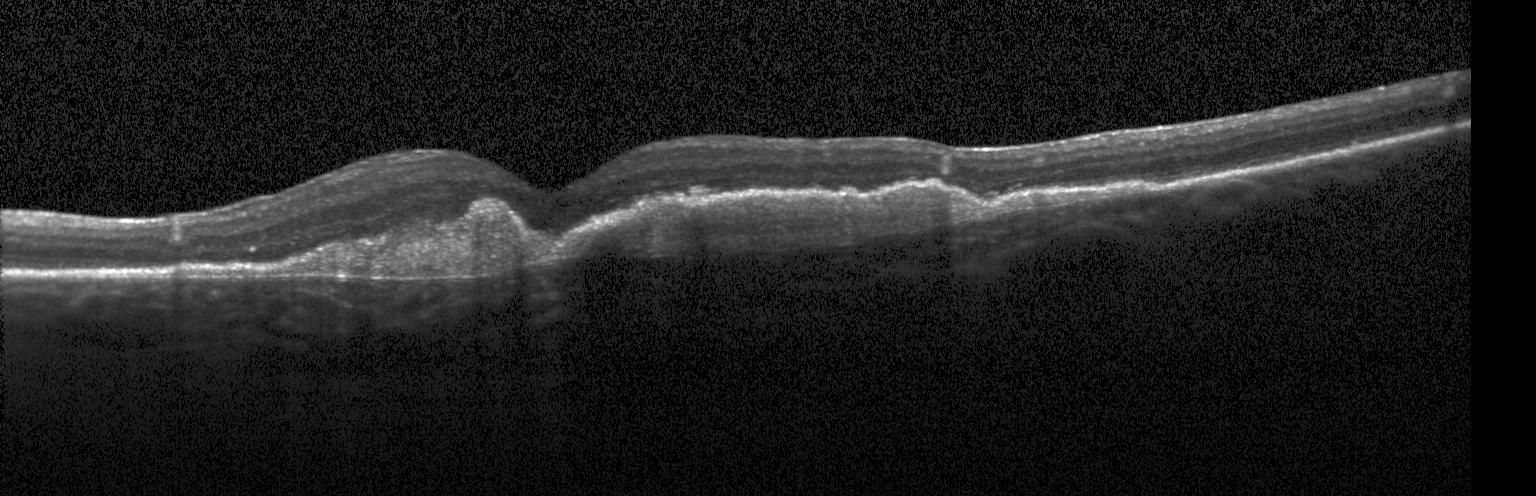

Heidelberg Spectralis · SD-OCT · macular scan · retinal OCT B-scan.
Finding: a choroidal neovascular membrane.